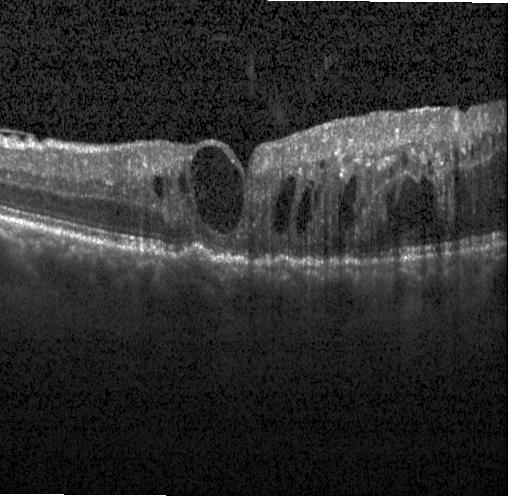

OCT finding: DME.